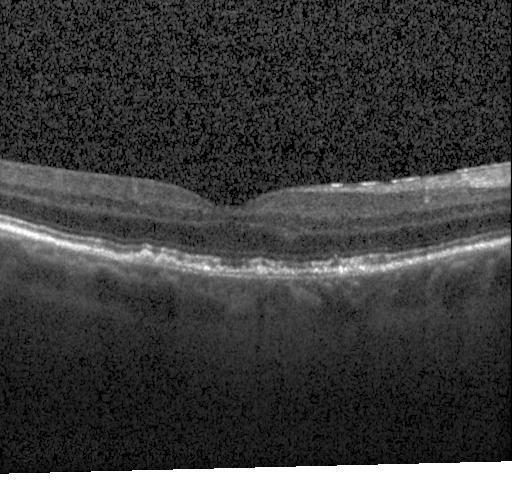
Instrument: Heidelberg Spectralis; OCT B-scan; SD-OCT. Assessment: multiple drusen.